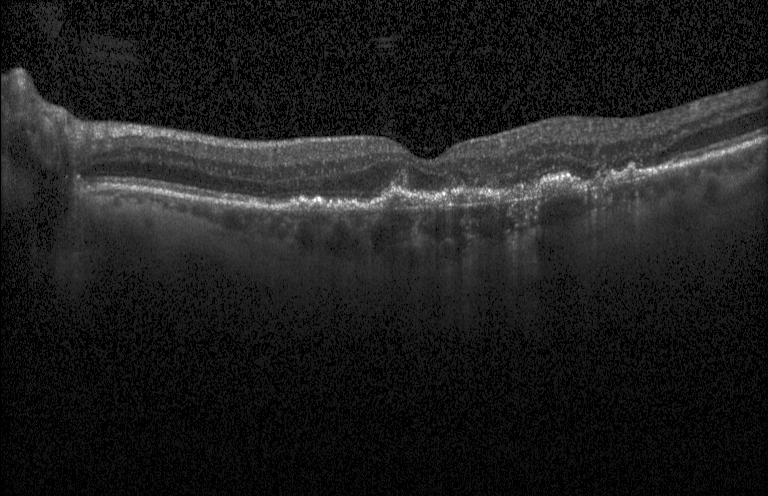
OCT B-scan showing a choroidal neovascular membrane.